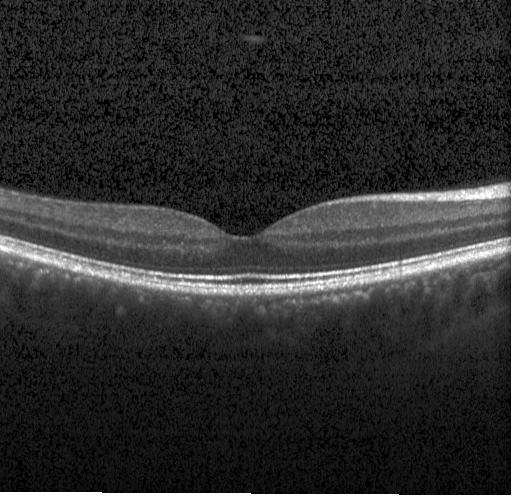

Retinal OCT B-scan — Assessment: no evidence of CNV, DME, or drusen.